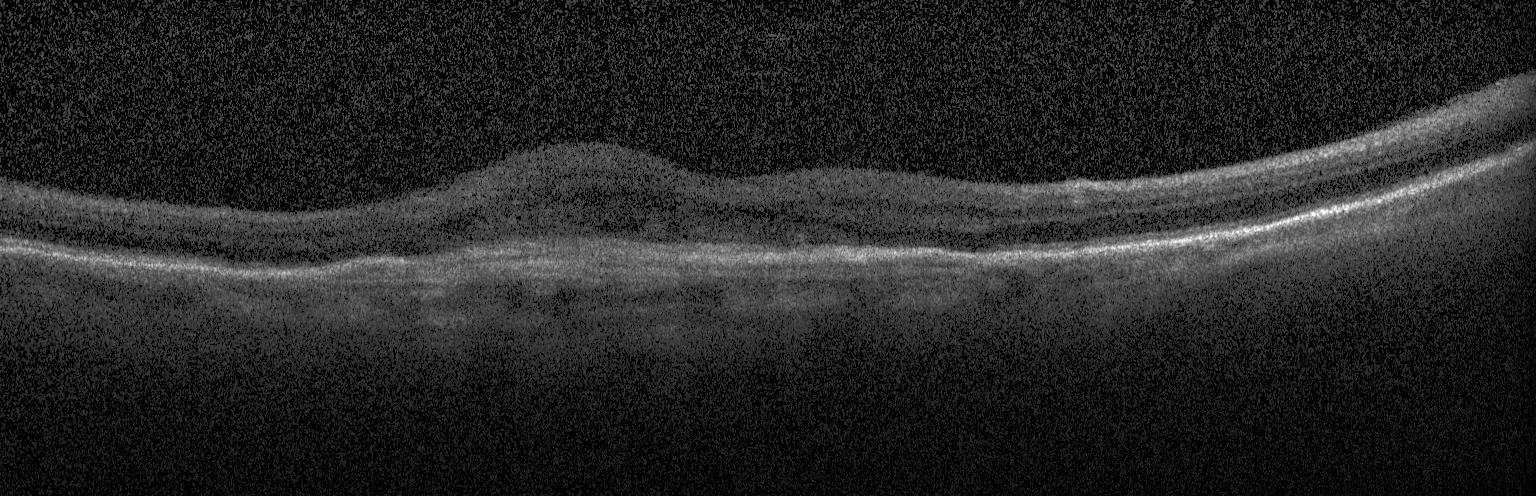
Diagnosis: choroidal neovascularization (CNV).